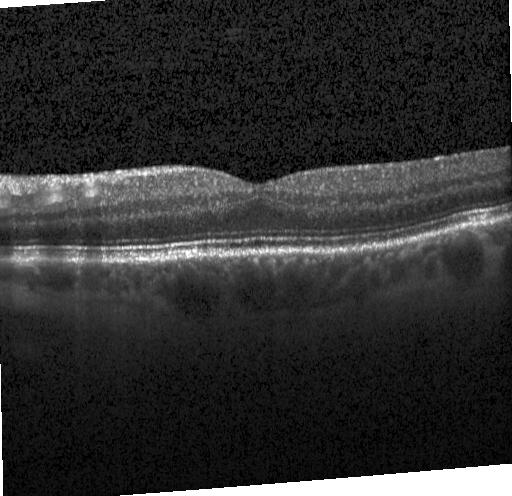
OCT B-scan; spectral-domain optical coherence tomography; horizontal scan through the fovea; acquired on a Heidelberg Spectralis. This B-scan demonstrates neither CNV, DME, nor drusen.